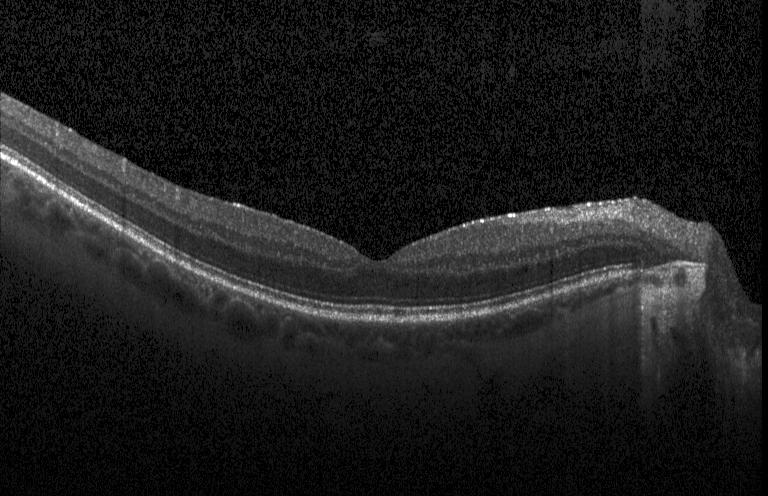

OCT line scan. Finding: no evidence of CNV, DME, or drusen.